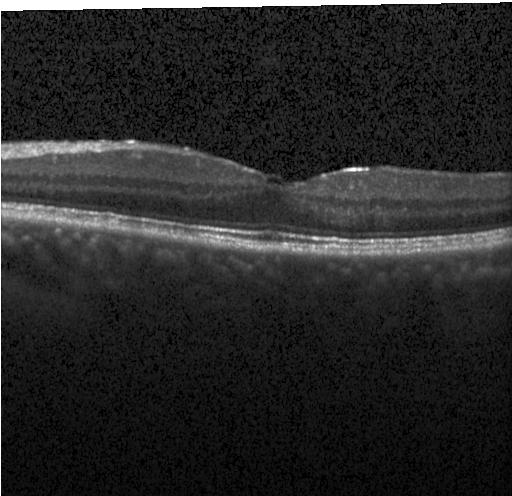
Through the macula; OCT B-scan; Heidelberg Spectralis; spectral-domain OCT
Impression: no choroidal neovascularization, no diabetic macular edema, and no drusen.